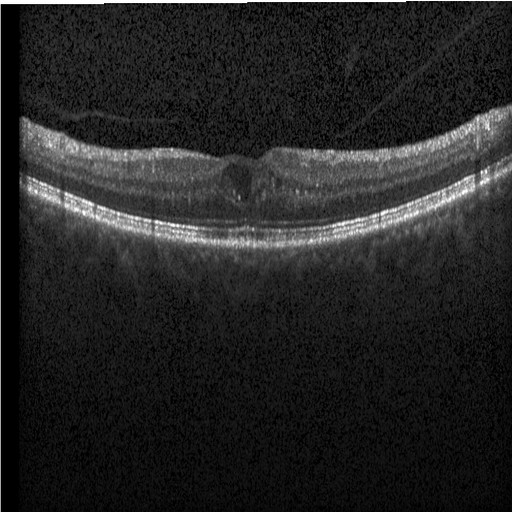
OCT finding: diabetic macular edema (DME).